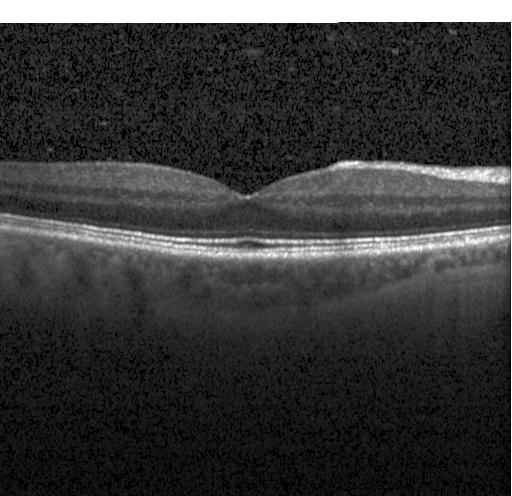
Spectral-domain OCT. Macular scan. OCT line scan — Diagnosis: neither CNV, DME, nor drusen.